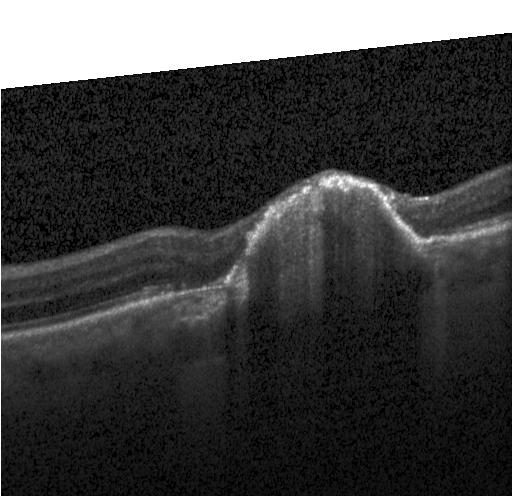

Centered on the fovea; SD-OCT; optical coherence tomography B-scan
Choroidal neovascularization.